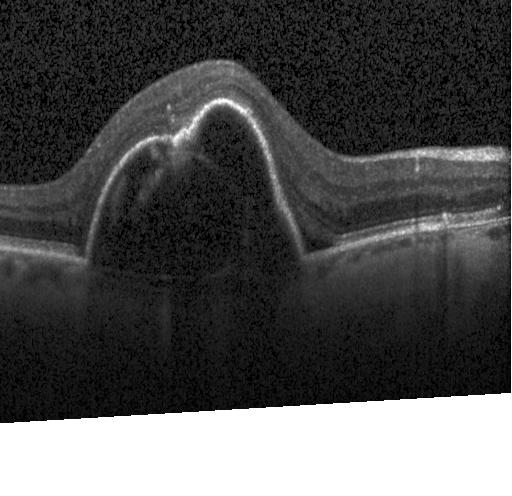 This B-scan demonstrates choroidal neovascularization.